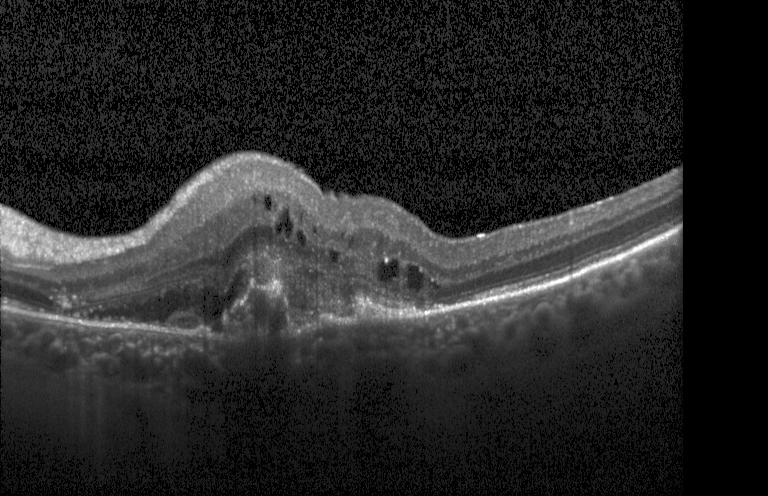 Optical coherence tomography B-scan. Diagnosis: a choroidal neovascular membrane.